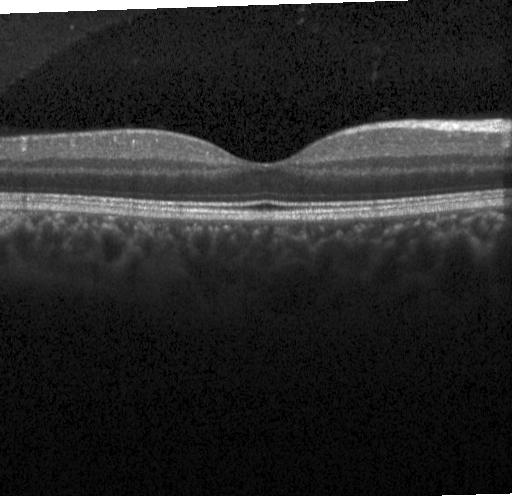

Retinal OCT B-scan — Diagnosis: no evidence of choroidal neovascularization, diabetic macular edema, or drusen.